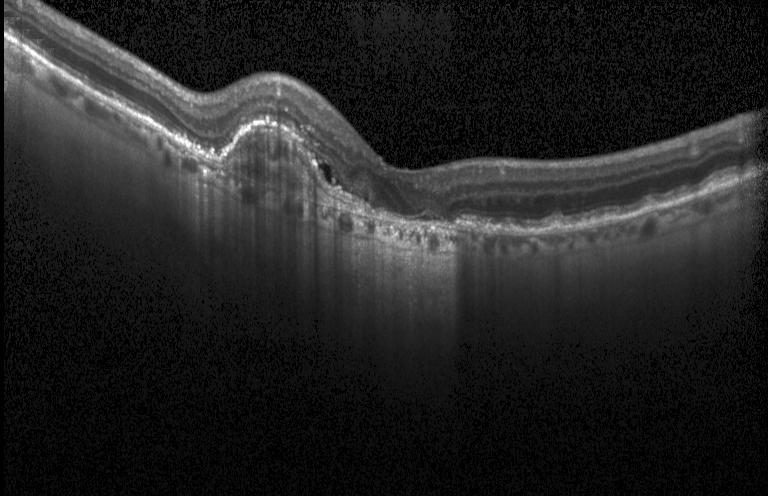
OCT B-scan, spectral-domain OCT. Impression: a choroidal neovascular membrane.